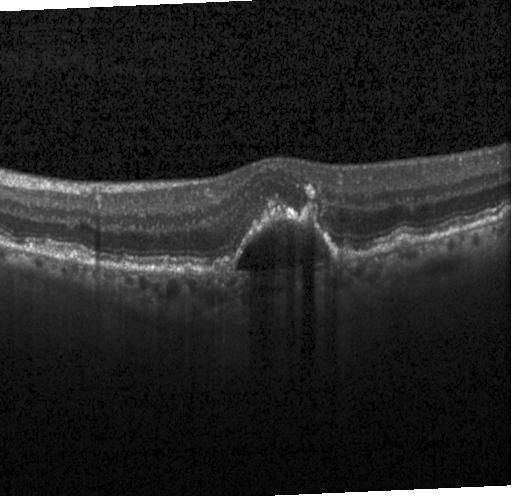 Optical coherence tomography scan. Macular OCT: choroidal neovascularization (CNV).